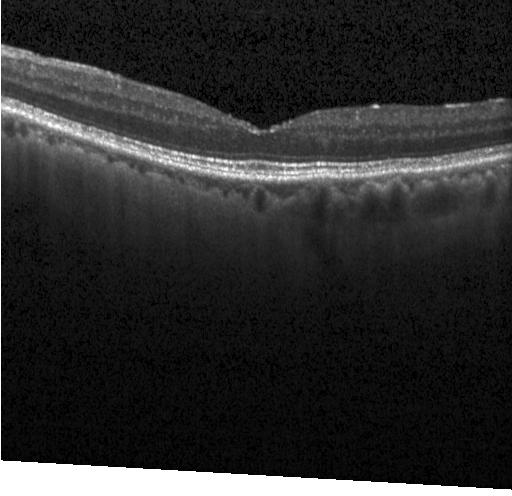
SD-OCT; fovea-centered; retinal OCT cross-section; Heidelberg Spectralis OCT system.
OCT finding: no evidence of choroidal neovascularization, diabetic macular edema, or drusen.